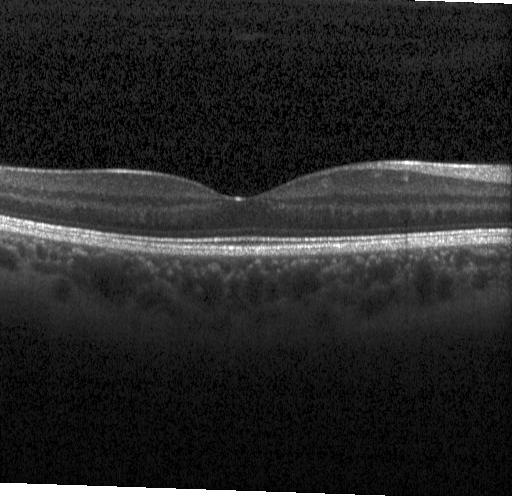
Macular OCT: no choroidal neovascularization, no diabetic macular edema, and no drusen.